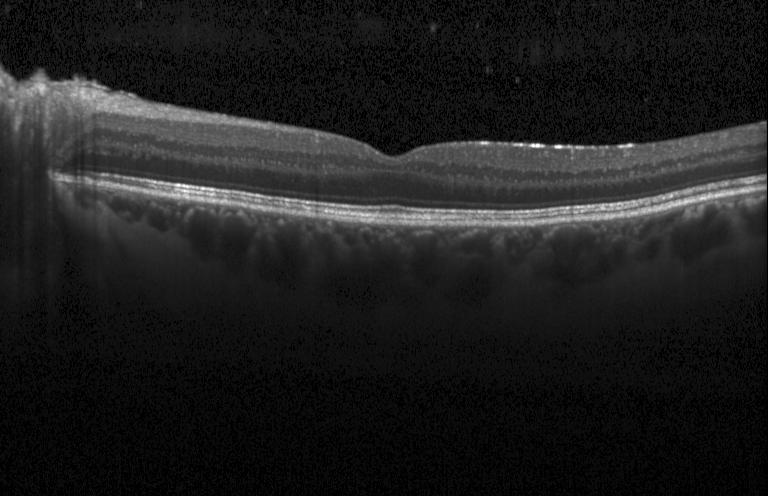 Retinal OCT B-scan, spectral-domain optical coherence tomography, acquired on a Heidelberg Spectralis — Impression: no choroidal neovascularization, no diabetic macular edema, and no drusen.